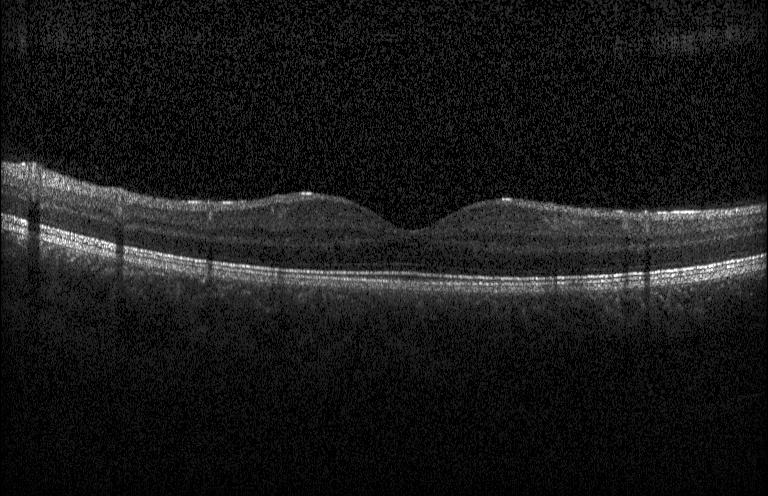

Optical coherence tomography B-scan
Assessment: neither choroidal neovascularization, diabetic macular edema, nor drusen.